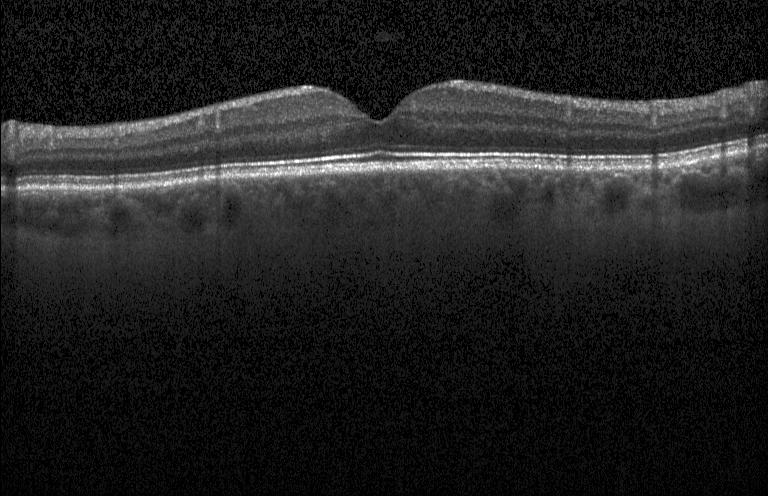
Spectral-domain OCT, macular scan, retinal OCT cross-section, instrument: Heidelberg Spectralis.
Finding: neither CNV, DME, nor drusen.